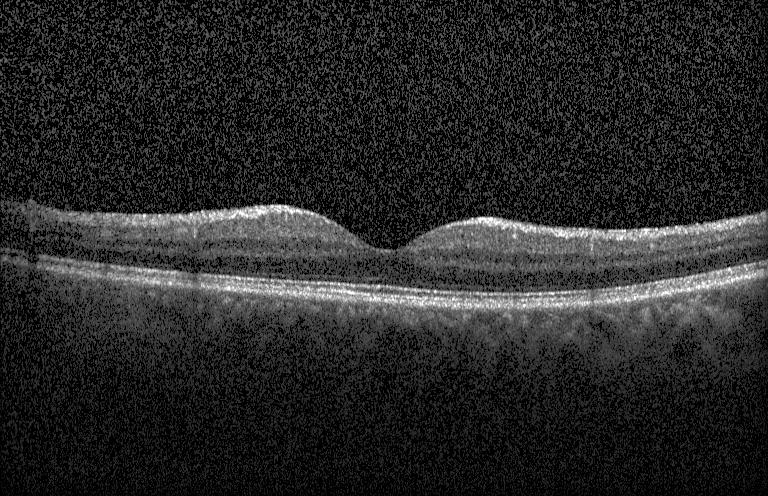 Acquired on a Heidelberg Spectralis. Through the macula. Retinal OCT cross-section. Spectral-domain OCT. Diagnosis: neither choroidal neovascularization, diabetic macular edema, nor drusen.